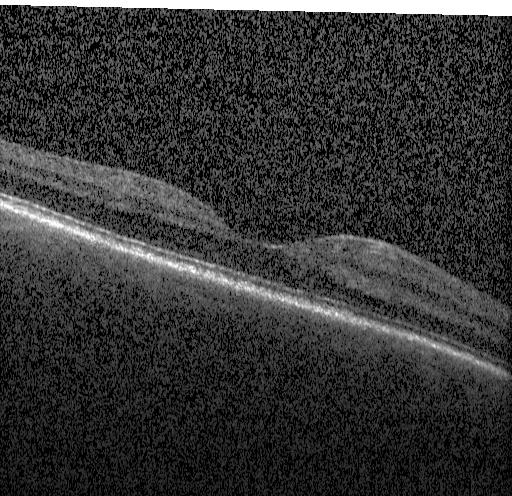
Fovea-centered; optical coherence tomography scan; Heidelberg Spectralis; spectral-domain optical coherence tomography.
This B-scan demonstrates no choroidal neovascularization, diabetic macular edema, or drusen.